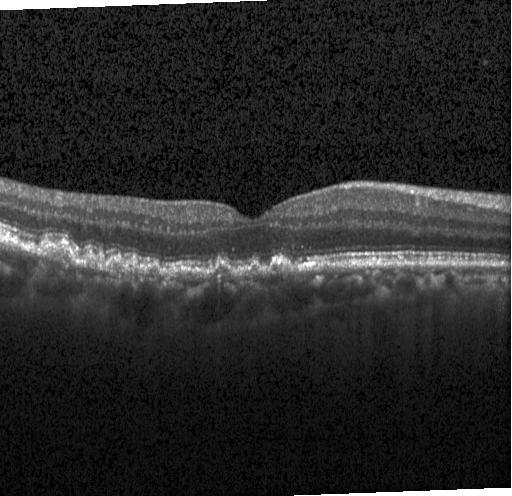 Optical coherence tomography B-scan · through the macula · Heidelberg Spectralis · spectral-domain OCT. Impression: sub-RPE drusenoid deposits.